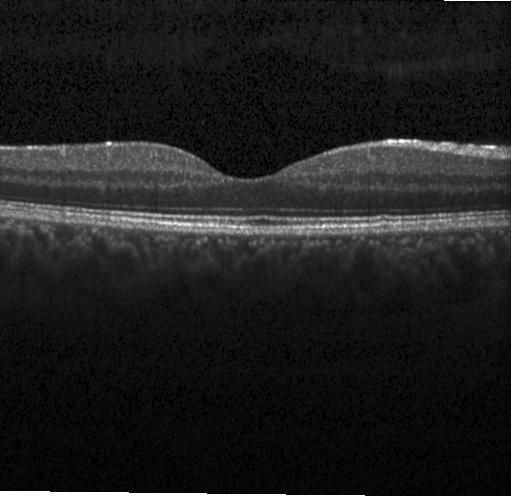
SD-OCT; retinal OCT B-scan; fovea-centered; instrument: Heidelberg Spectralis. Diagnosis: neither choroidal neovascularization, diabetic macular edema, nor drusen.